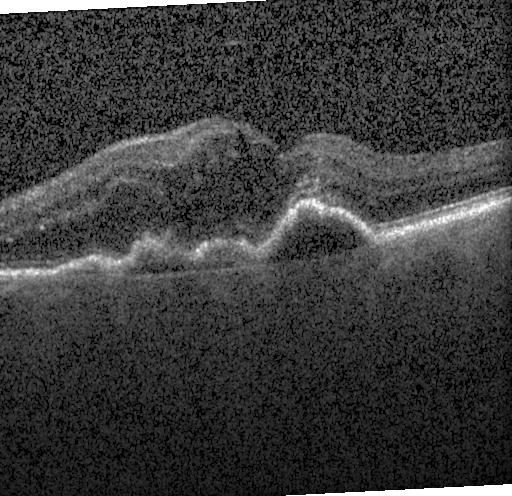

Instrument: Heidelberg Spectralis; spectral-domain OCT; OCT B-scan; centered on the fovea.
Assessment: choroidal neovascularization.